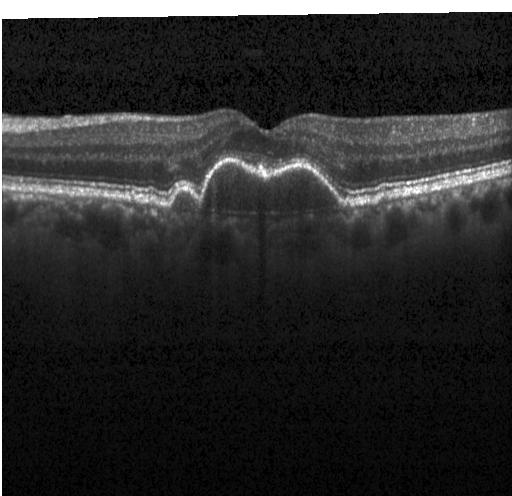
Heidelberg Spectralis. Through the macula. Optical coherence tomography B-scan
Assessment: CNV.